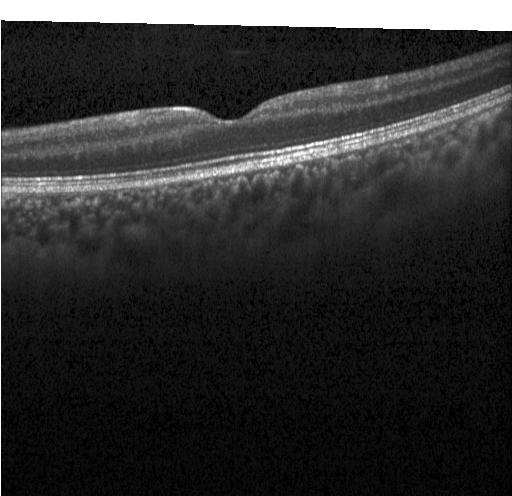 Heidelberg Spectralis · SD-OCT · OCT line scan · macular scan. The scan shows neither CNV, DME, nor drusen.